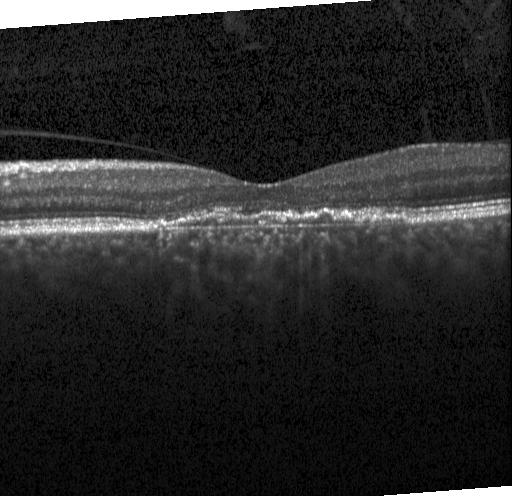
Retinal OCT B-scan. Spectral-domain optical coherence tomography. Centered on the fovea. Instrument: Heidelberg Spectralis. This B-scan demonstrates CNV.